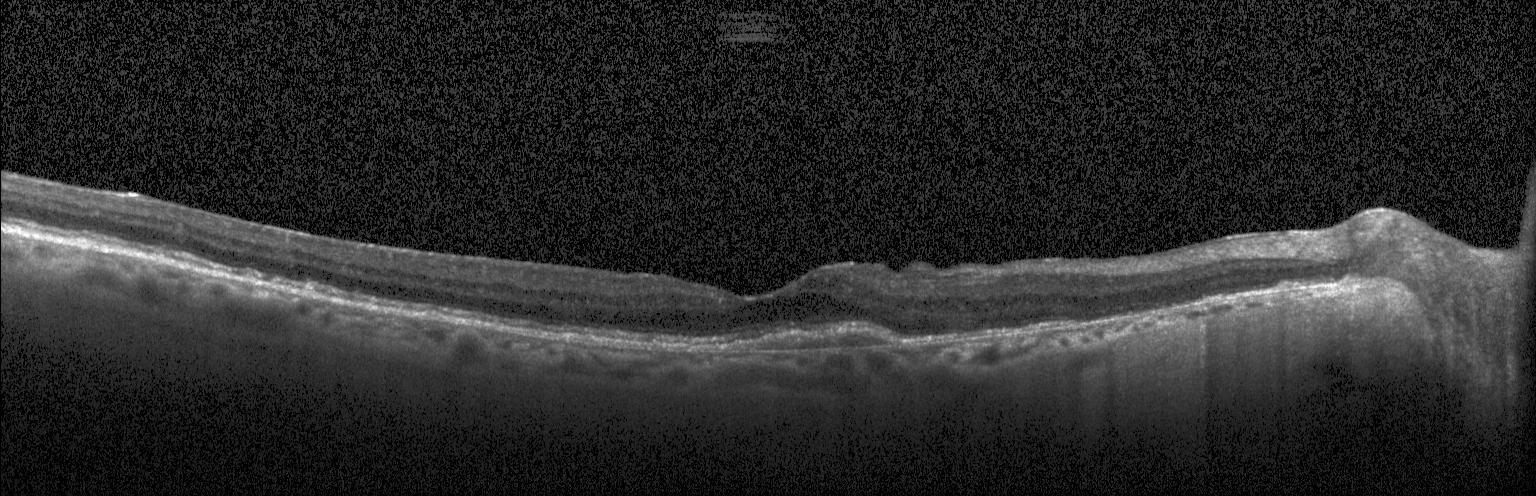 Retinal OCT cross-section, horizontal scan through the fovea, acquired on a Heidelberg Spectralis, spectral-domain optical coherence tomography.
Dx: choroidal neovascularization (CNV).